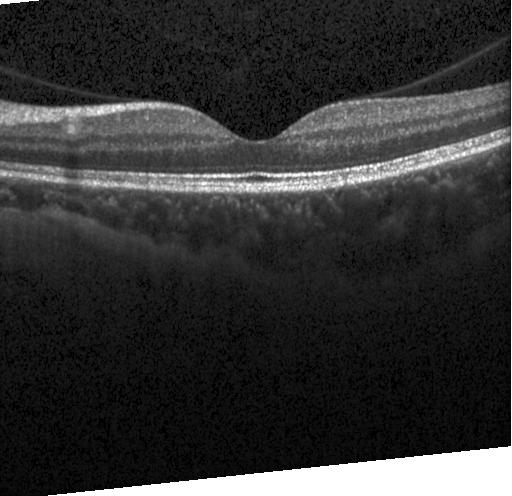

Spectral-domain optical coherence tomography, optical coherence tomography scan, Heidelberg Spectralis, through the macula
Neither CNV, DME, nor drusen.